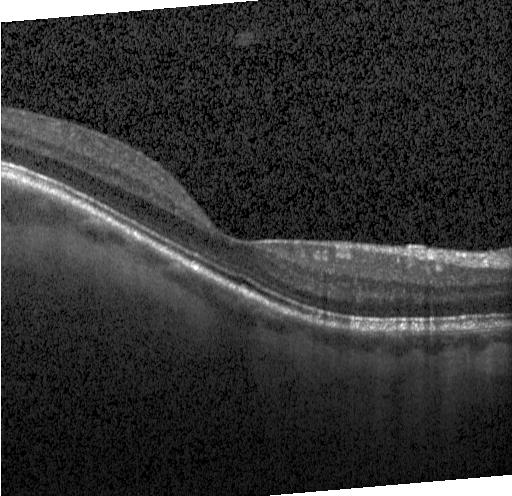
OCT scan showing no evidence of choroidal neovascularization, diabetic macular edema, or drusen.